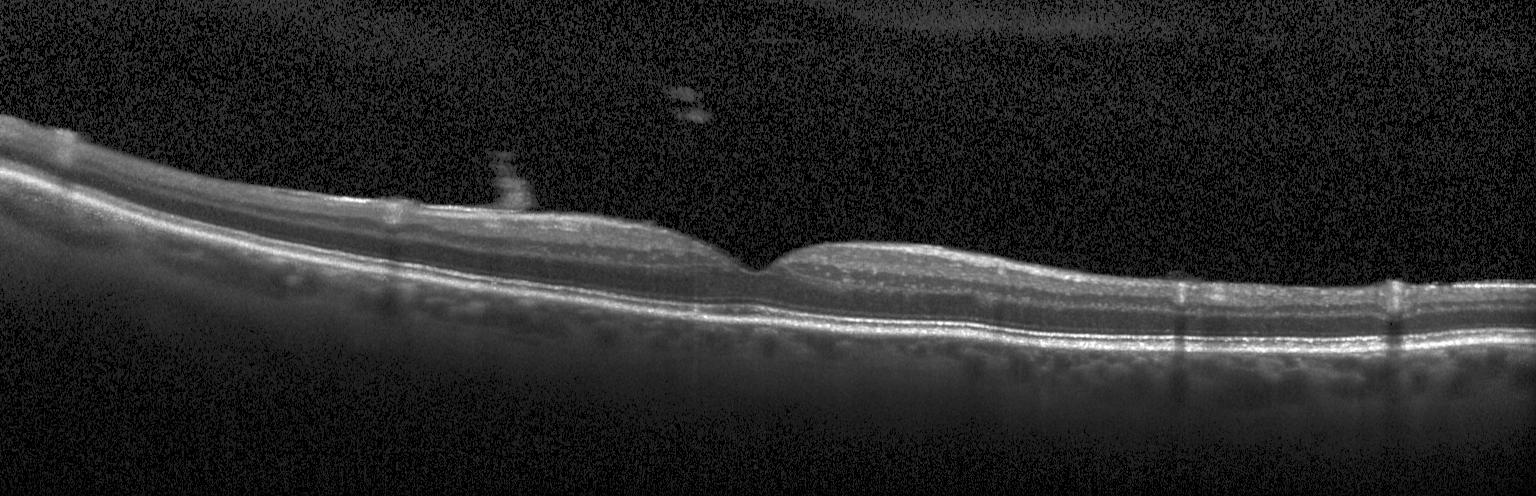 Spectral-domain OCT · Heidelberg Spectralis · retinal OCT B-scan · through the macula — Impression: no choroidal neovascularization, diabetic macular edema, or drusen.